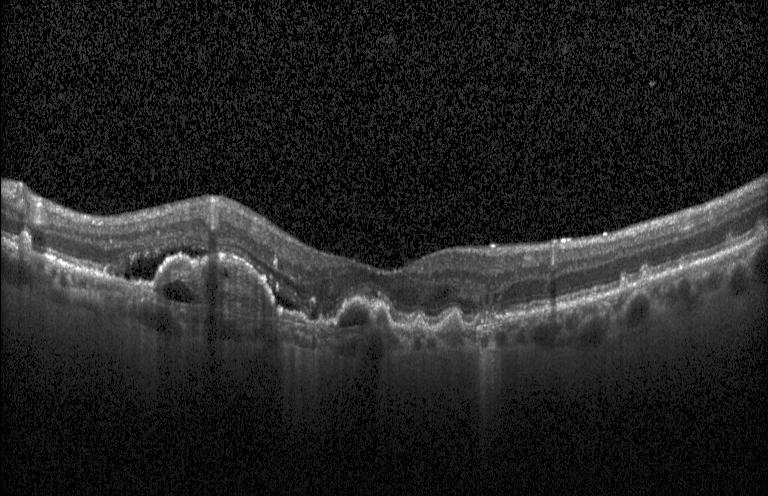 SD-OCT · horizontal scan through the fovea · Heidelberg Spectralis · optical coherence tomography B-scan.
This B-scan demonstrates choroidal neovascularization.